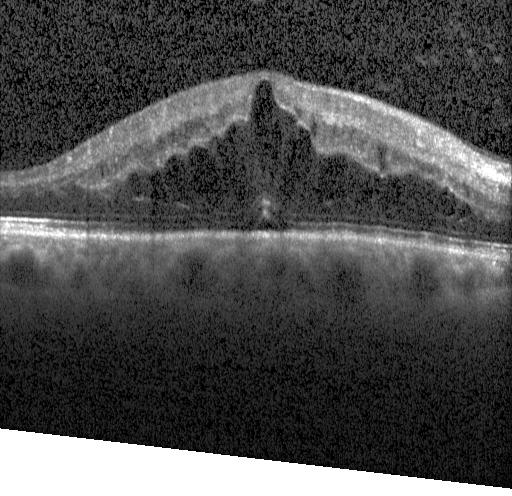 Retinal OCT B-scan
Diagnosis: diabetic macular edema.